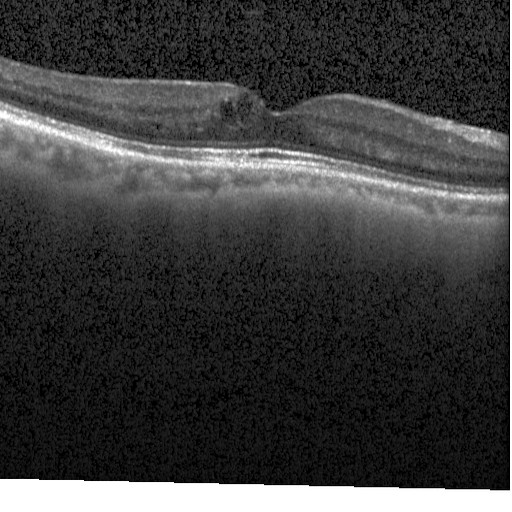

OCT line scan. Macular OCT: diabetic macular edema.